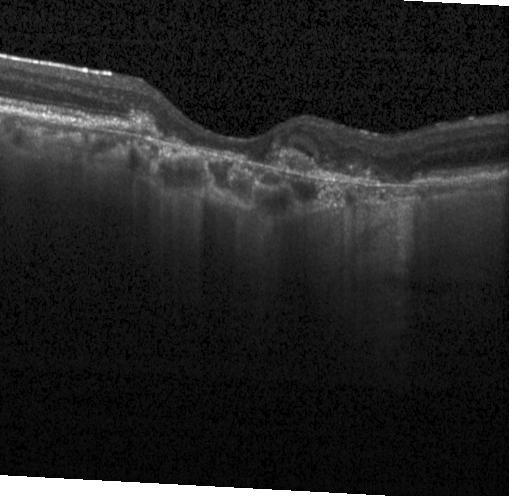
OCT B-scan.
Macular OCT: a choroidal neovascular membrane.